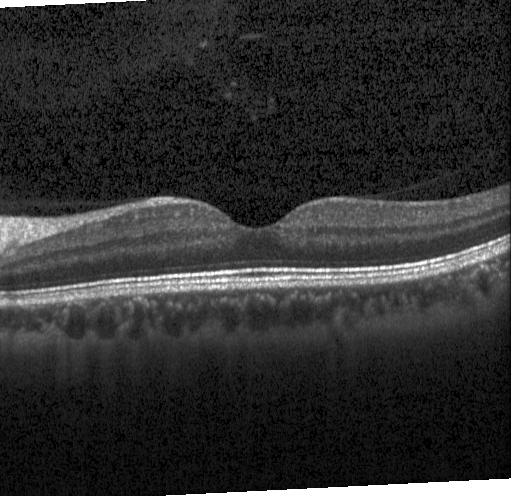 Spectral-domain optical coherence tomography · OCT line scan · Heidelberg Spectralis OCT system. Impression: no CNV, no DME, and no drusen.